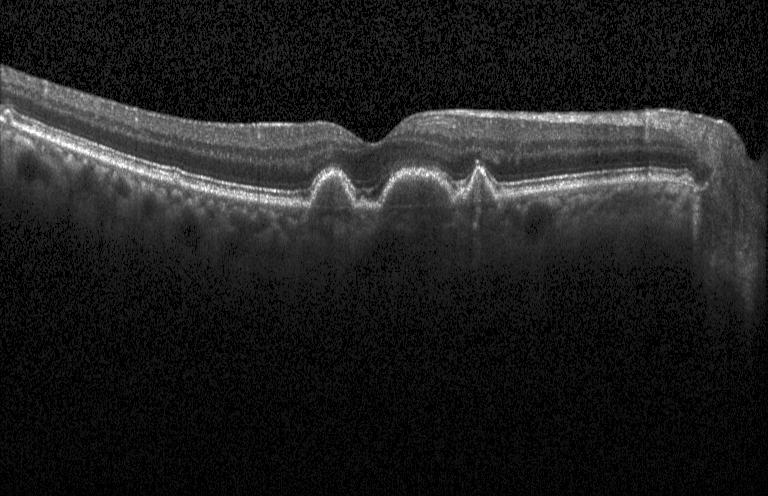
OCT line scan — Impression: multiple drusen.